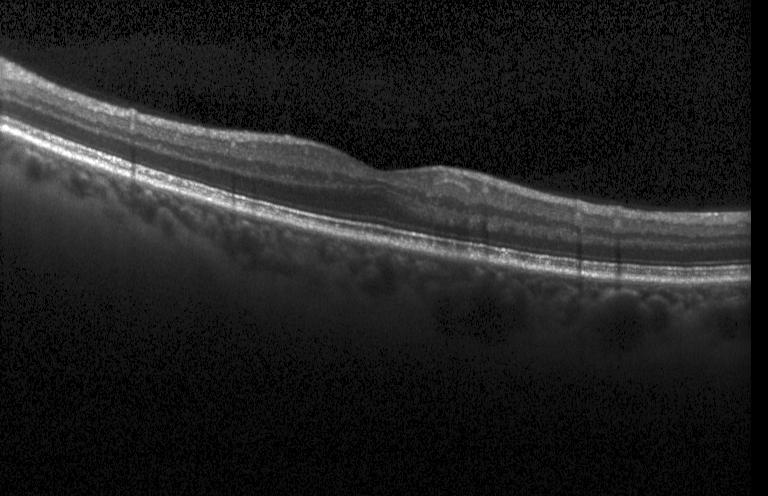
Horizontal scan through the fovea. Retinal OCT cross-section. Heidelberg Spectralis OCT system
Macular OCT: no CNV, no DME, and no drusen.